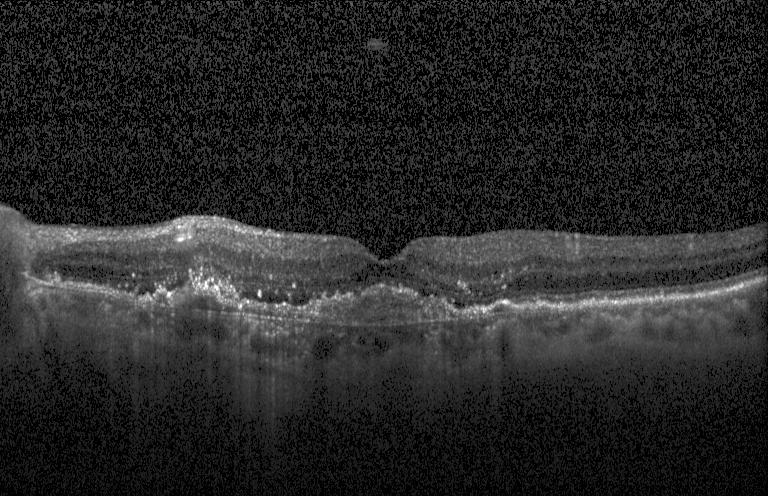
Dx: choroidal neovascularization (CNV).